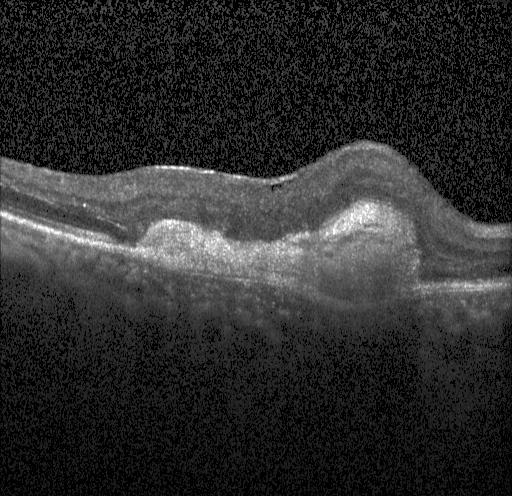

OCT line scan. Through the macula
Assessment: a choroidal neovascular membrane.